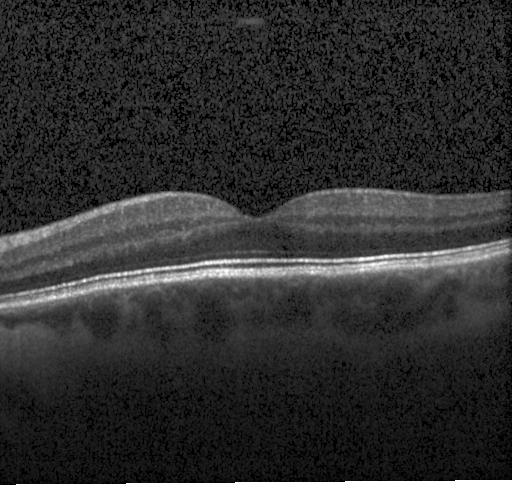

No CNV, DME, or drusen.